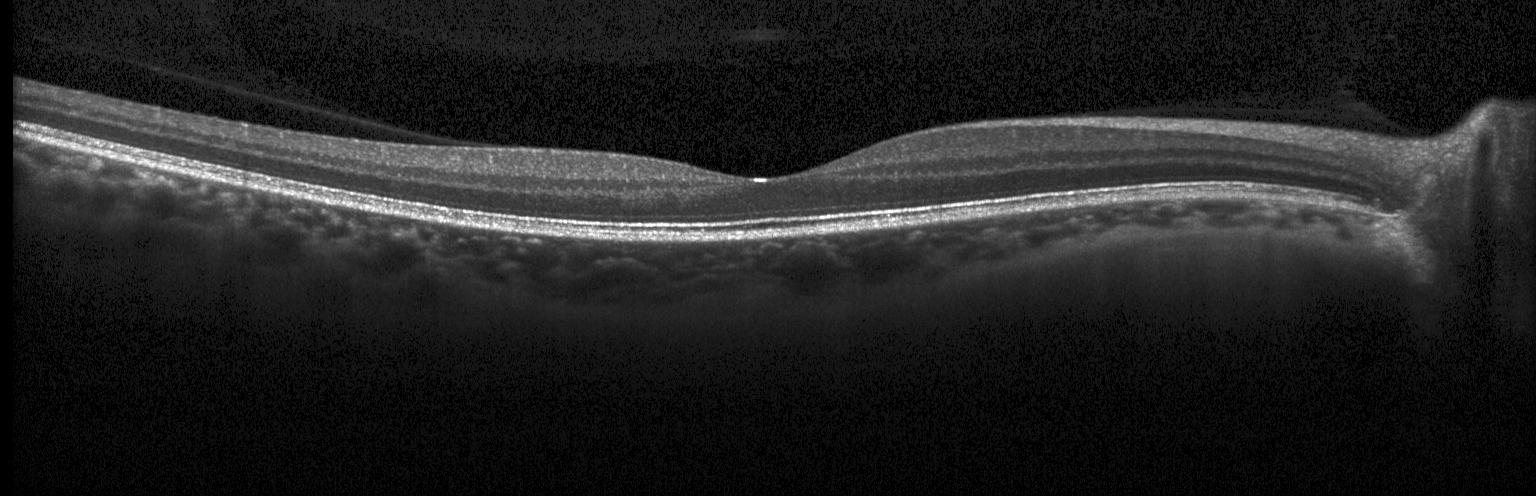
Finding: neither choroidal neovascularization, diabetic macular edema, nor drusen.